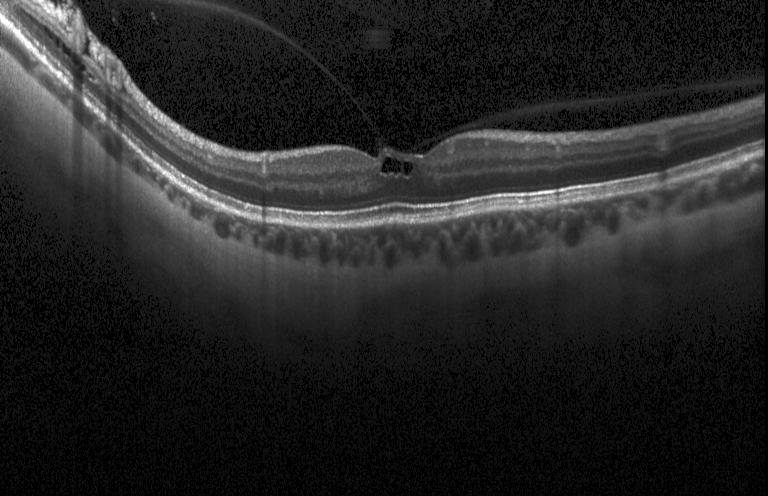 Heidelberg Spectralis OCT system; optical coherence tomography B-scan; spectral-domain OCT; horizontal scan through the fovea.
Impression: neither choroidal neovascularization, diabetic macular edema, nor drusen.